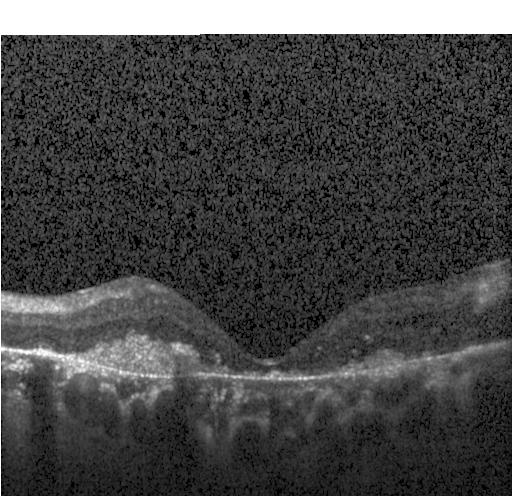

Finding: a choroidal neovascular membrane.